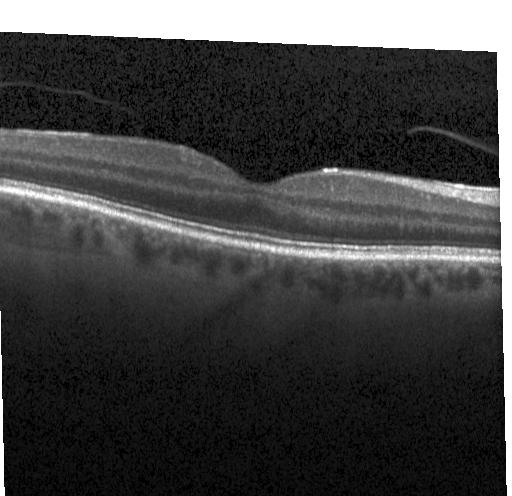
Horizontal scan through the fovea · OCT line scan · Heidelberg Spectralis OCT system
Impression: neither choroidal neovascularization, diabetic macular edema, nor drusen.